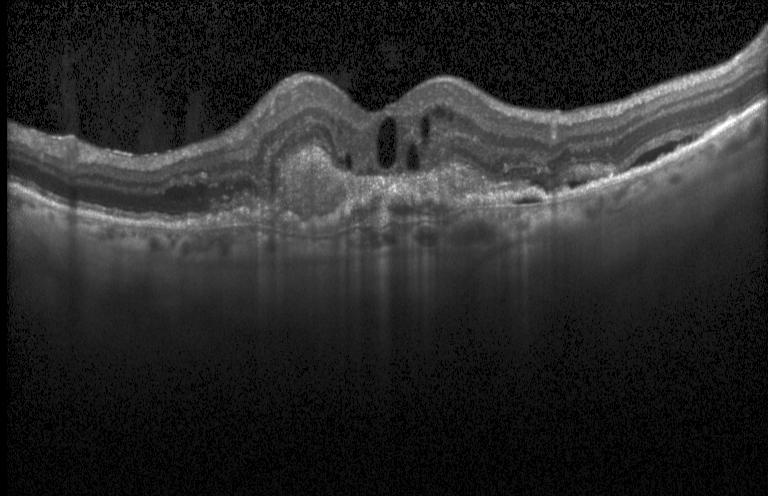
Finding: a choroidal neovascular membrane.